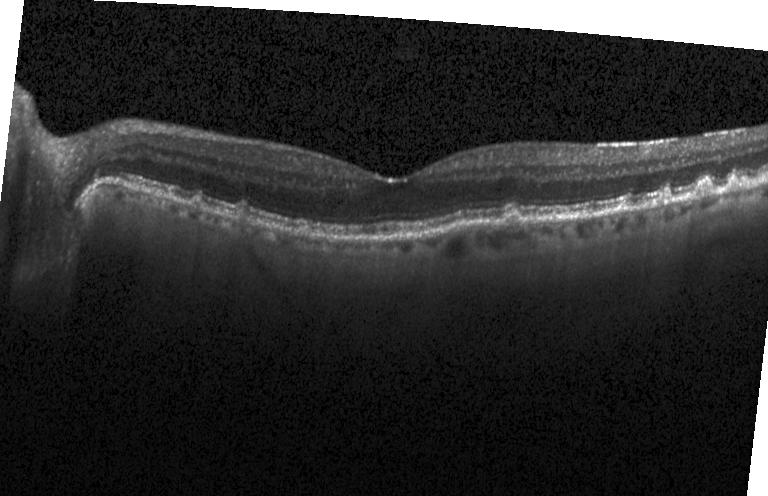
Retinal OCT cross-section. Acquired on a Heidelberg Spectralis.
Finding: sub-RPE drusenoid deposits.